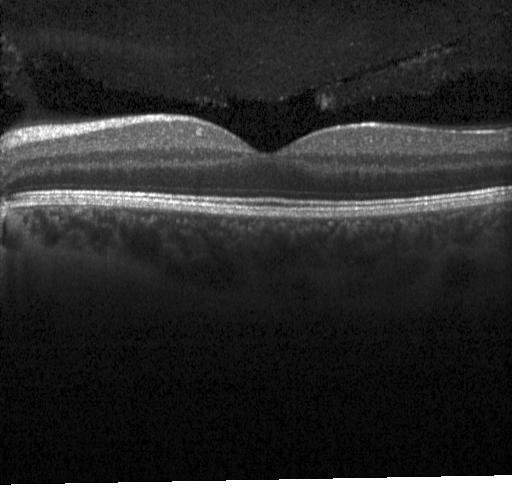
Dx: neither choroidal neovascularization, diabetic macular edema, nor drusen.